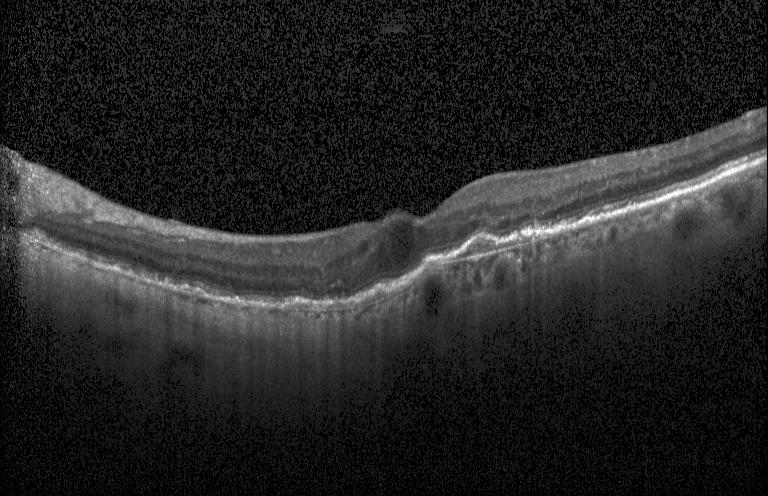
Spectral-domain optical coherence tomography, centered on the fovea, Heidelberg Spectralis OCT system, OCT B-scan.
Dx: choroidal neovascularization (CNV).